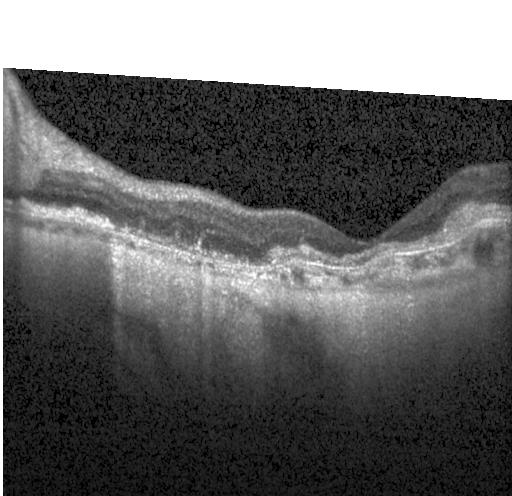
Fovea-centered. Retinal OCT cross-section. SD-OCT. Impression: choroidal neovascularization.